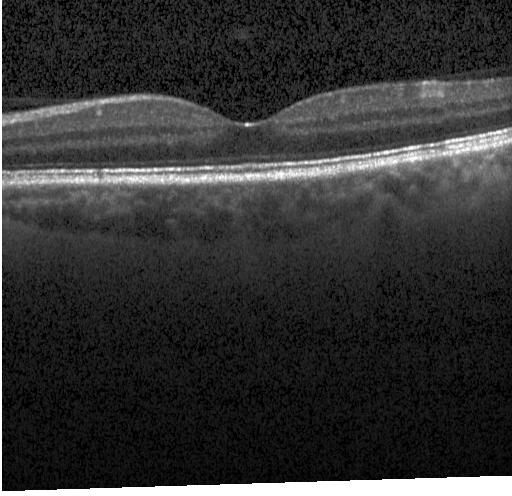 Acquired on a Heidelberg Spectralis · spectral-domain OCT · OCT line scan — Diagnosis: neither choroidal neovascularization, diabetic macular edema, nor drusen.